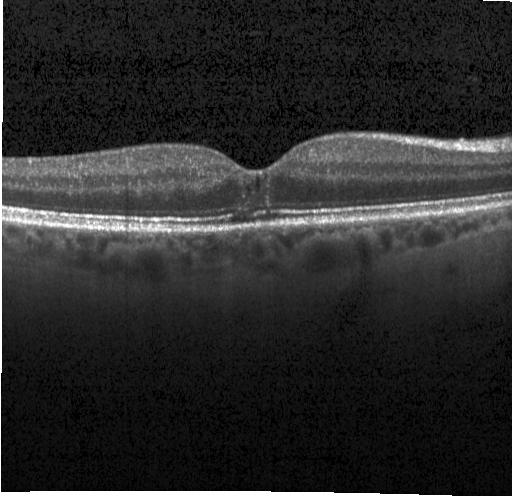
Retinal OCT B-scan, spectral-domain optical coherence tomography — Diagnosis: no evidence of choroidal neovascularization, diabetic macular edema, or drusen.